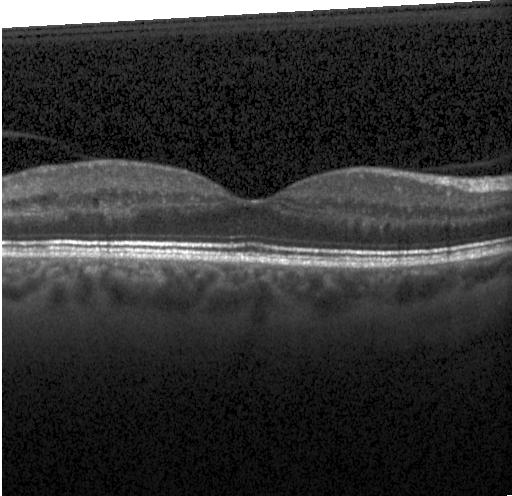 OCT B-scan — Impression: DME.